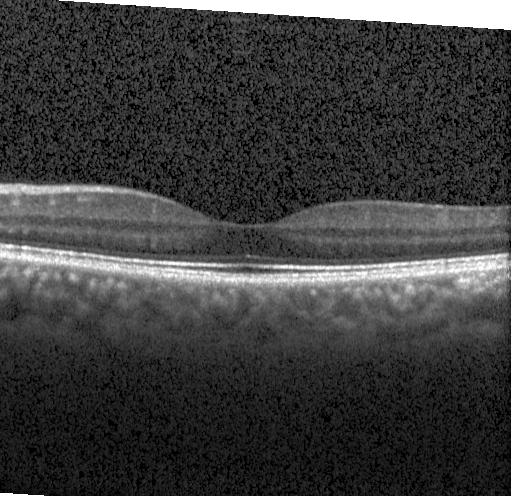 Finding: neither CNV, DME, nor drusen.